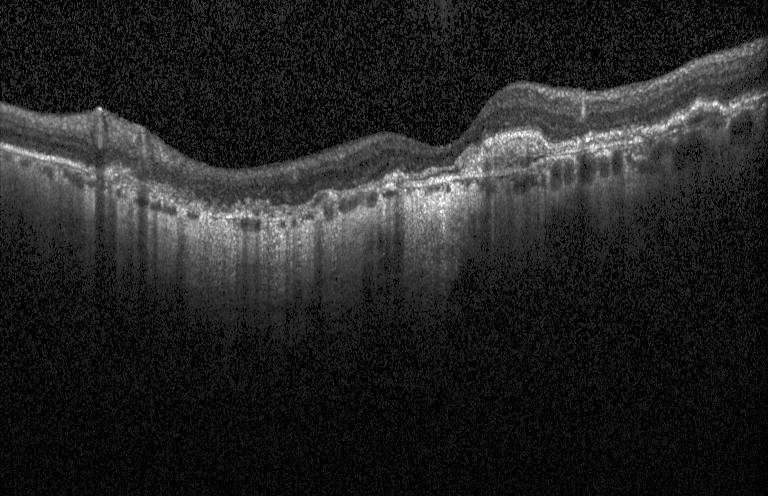
Finding: a choroidal neovascular membrane.